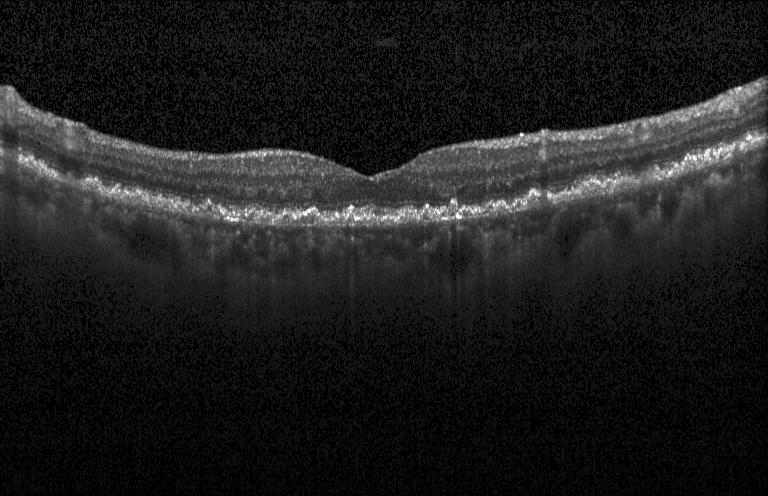

Drusen.